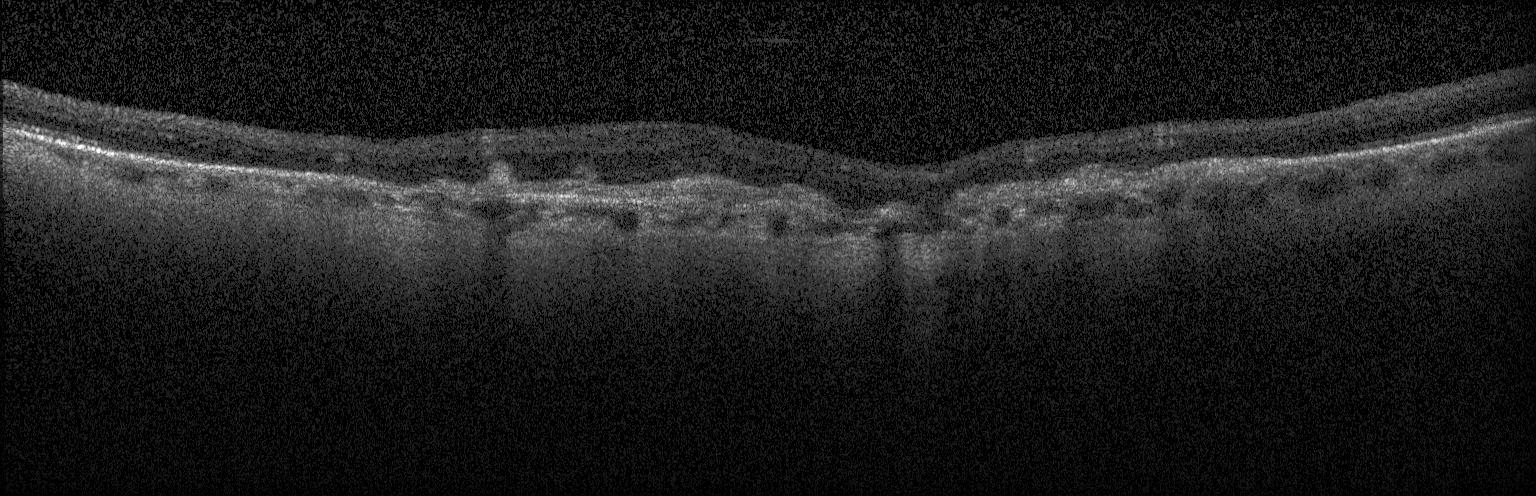

Diagnosis: a choroidal neovascular membrane.